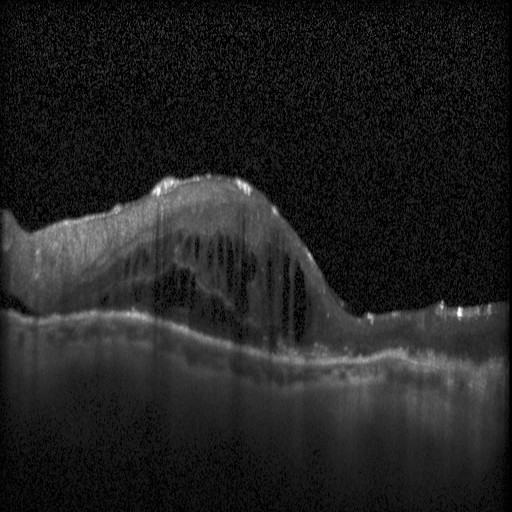
Finding: diabetic macular edema.